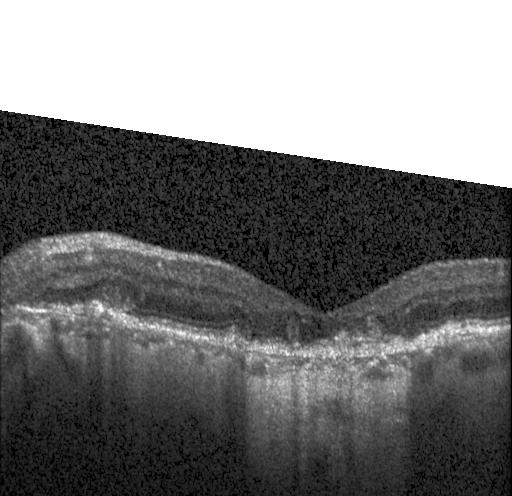
Heidelberg Spectralis; OCT line scan.
This B-scan demonstrates a choroidal neovascular membrane.